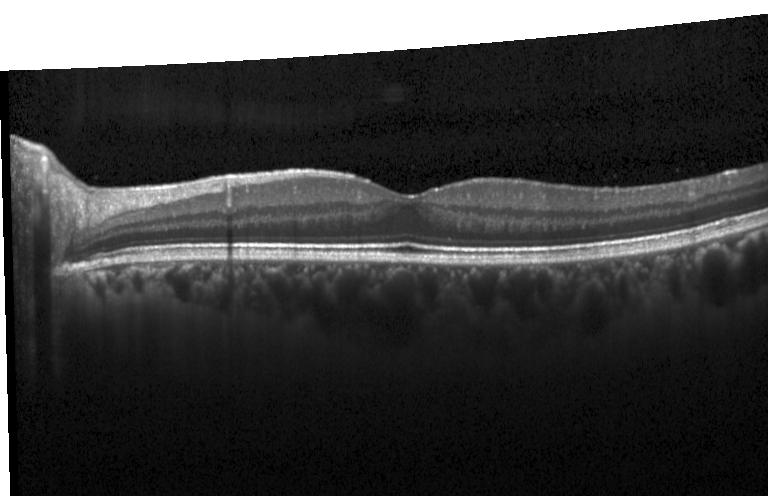 Retinal OCT B-scan
Finding: no choroidal neovascularization, no diabetic macular edema, and no drusen.